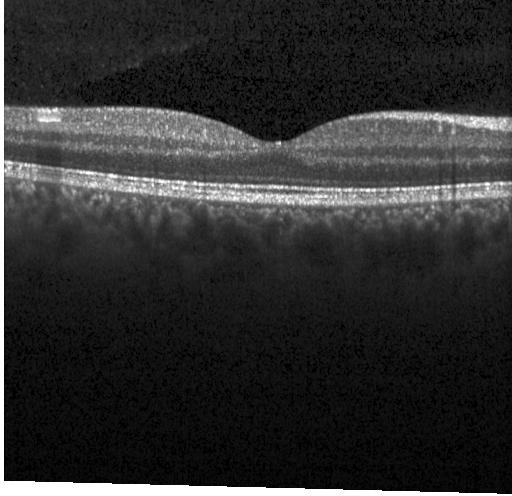 OCT B-scan. Acquired on a Heidelberg Spectralis. Spectral-domain OCT.
No choroidal neovascularization, no diabetic macular edema, and no drusen.